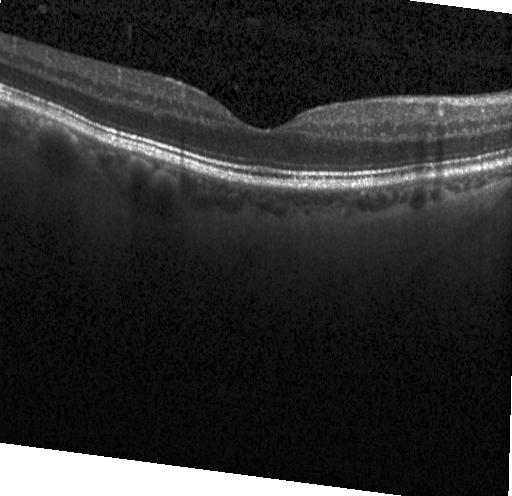 Spectral-domain OCT B-scan: neither choroidal neovascularization, diabetic macular edema, nor drusen.